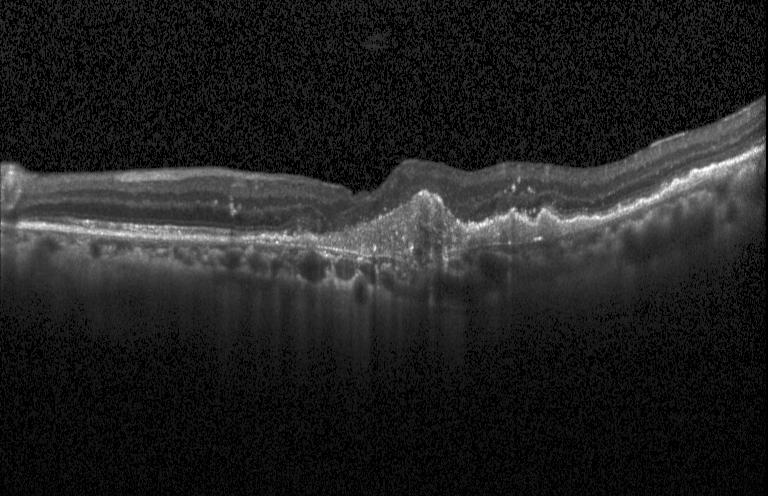 SD-OCT · centered on the fovea · retinal OCT cross-section · Heidelberg Spectralis.
The scan shows a choroidal neovascular membrane.